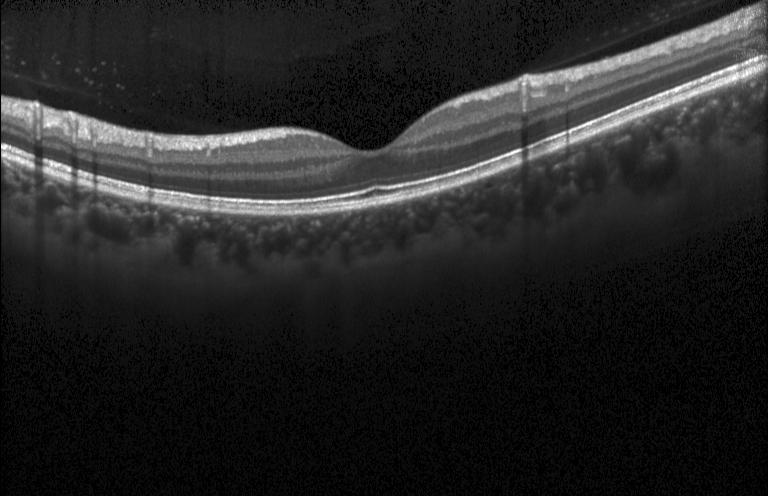

OCT scan showing no evidence of CNV, DME, or drusen.